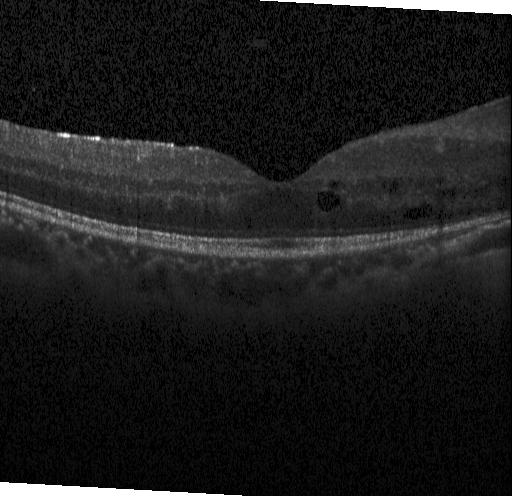
Centered on the fovea, OCT B-scan, SD-OCT — This B-scan demonstrates diabetic macular edema (DME).